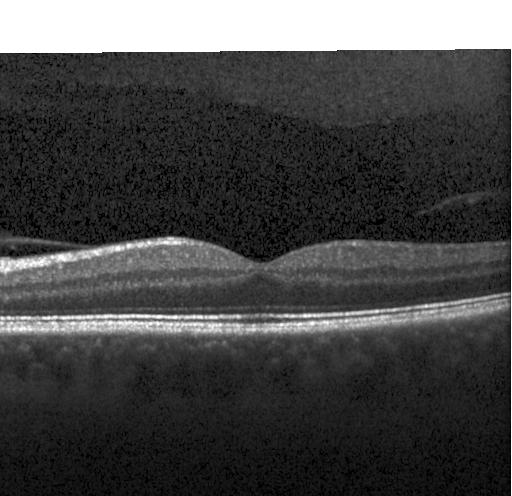 Spectral-domain optical coherence tomography · instrument: Heidelberg Spectralis · fovea-centered · retinal OCT cross-section.
Macular OCT: no CNV, DME, or drusen.